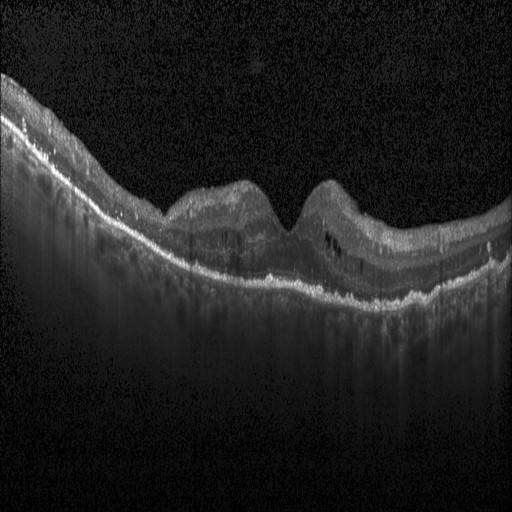

Optical coherence tomography scan
Finding: DME.